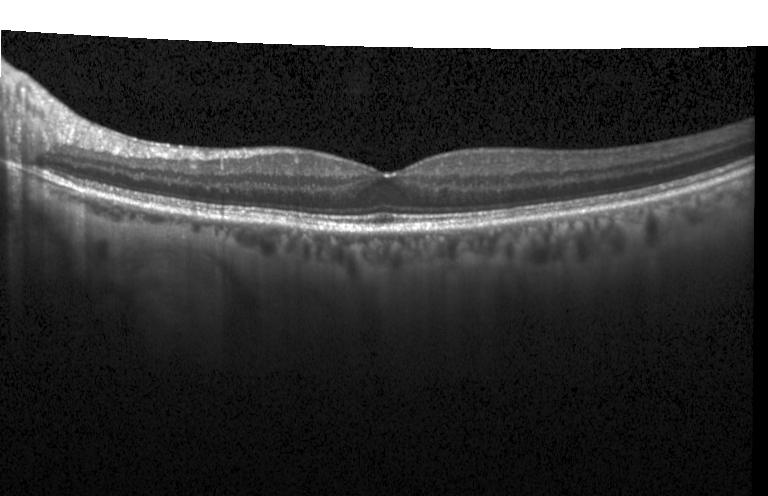

Macular OCT: no evidence of choroidal neovascularization, diabetic macular edema, or drusen.